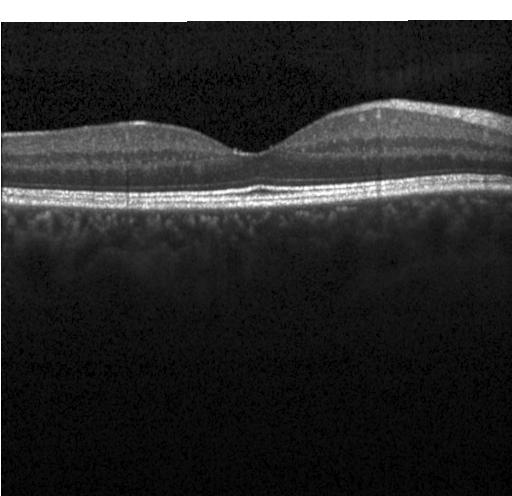 Spectral-domain optical coherence tomography, Heidelberg Spectralis OCT system, OCT B-scan. Impression: no evidence of CNV, DME, or drusen.